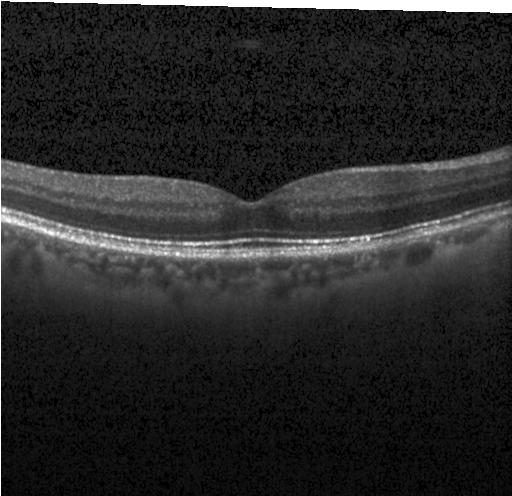 This B-scan demonstrates no choroidal neovascularization, no diabetic macular edema, and no drusen.